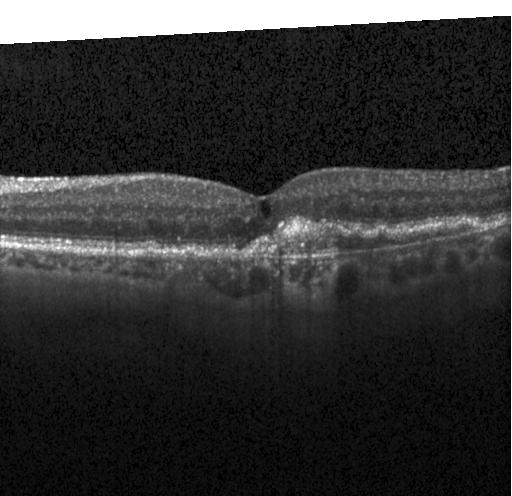
Impression: choroidal neovascularization.